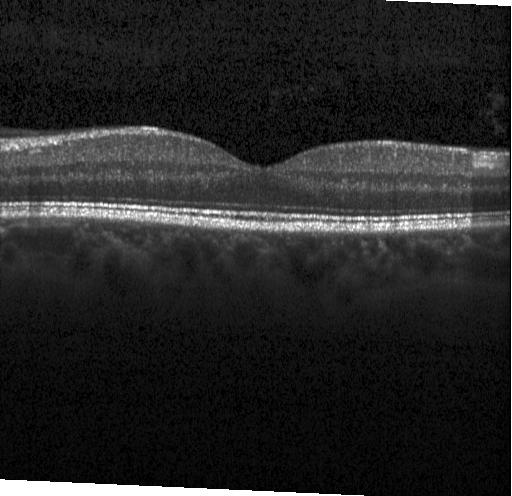
Horizontal scan through the fovea, optical coherence tomography scan.
Finding: no choroidal neovascularization, no diabetic macular edema, and no drusen.